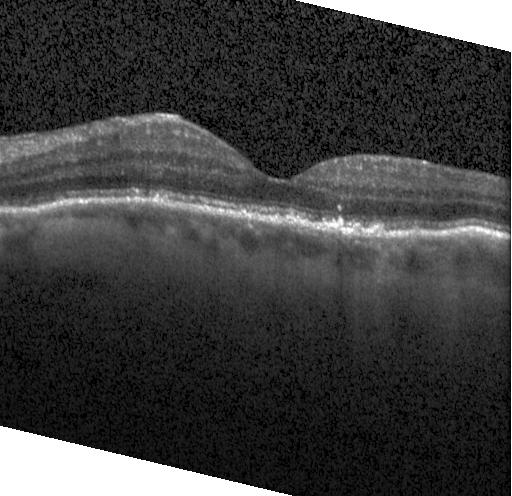
Through the macula. Retinal OCT B-scan. Spectral-domain optical coherence tomography — OCT finding: sub-RPE drusenoid deposits.